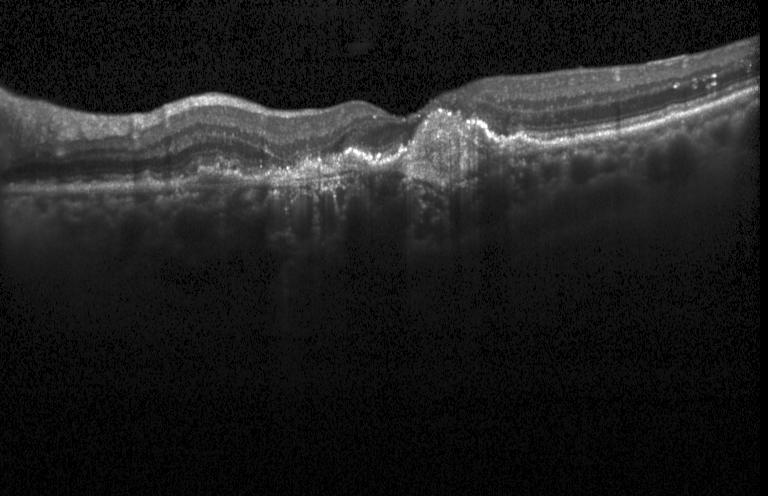 OCT finding: a choroidal neovascular membrane.